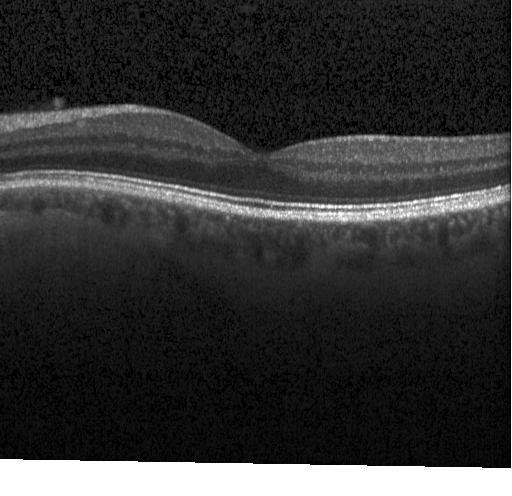

OCT finding: no choroidal neovascularization, no diabetic macular edema, and no drusen.